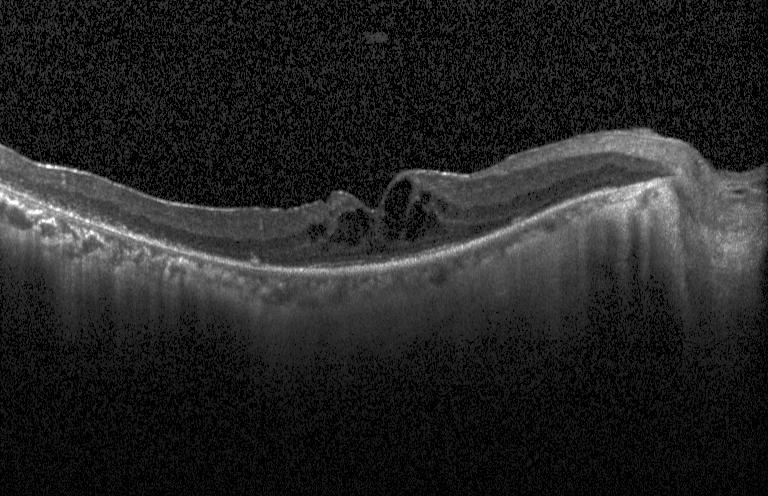
OCT B-scan showing diabetic macular edema (DME).